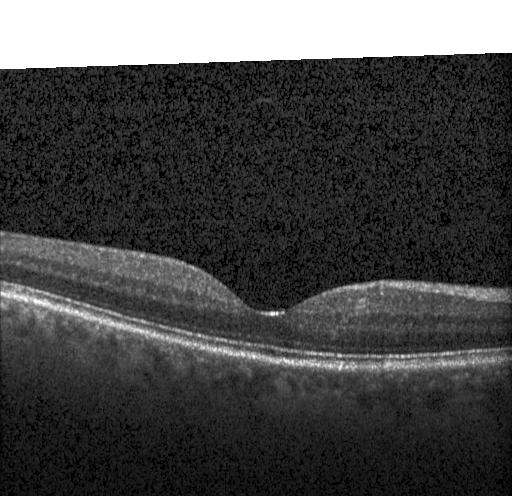 Retinal OCT cross-section — Diagnosis: no choroidal neovascularization, diabetic macular edema, or drusen.